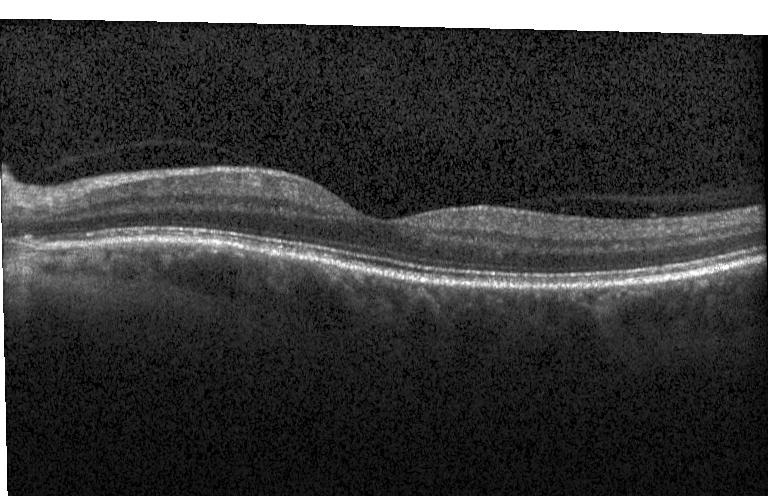

Spectral-domain optical coherence tomography, Heidelberg Spectralis, OCT B-scan
OCT finding: no CNV, no DME, and no drusen.